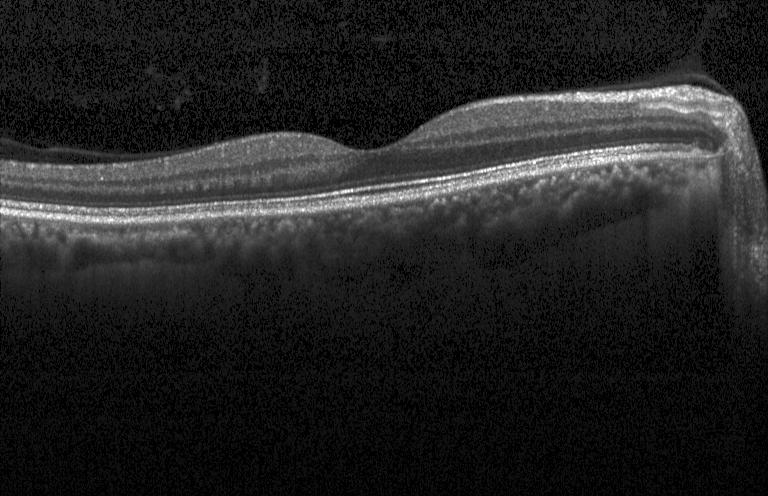

Impression: no choroidal neovascularization, diabetic macular edema, or drusen.